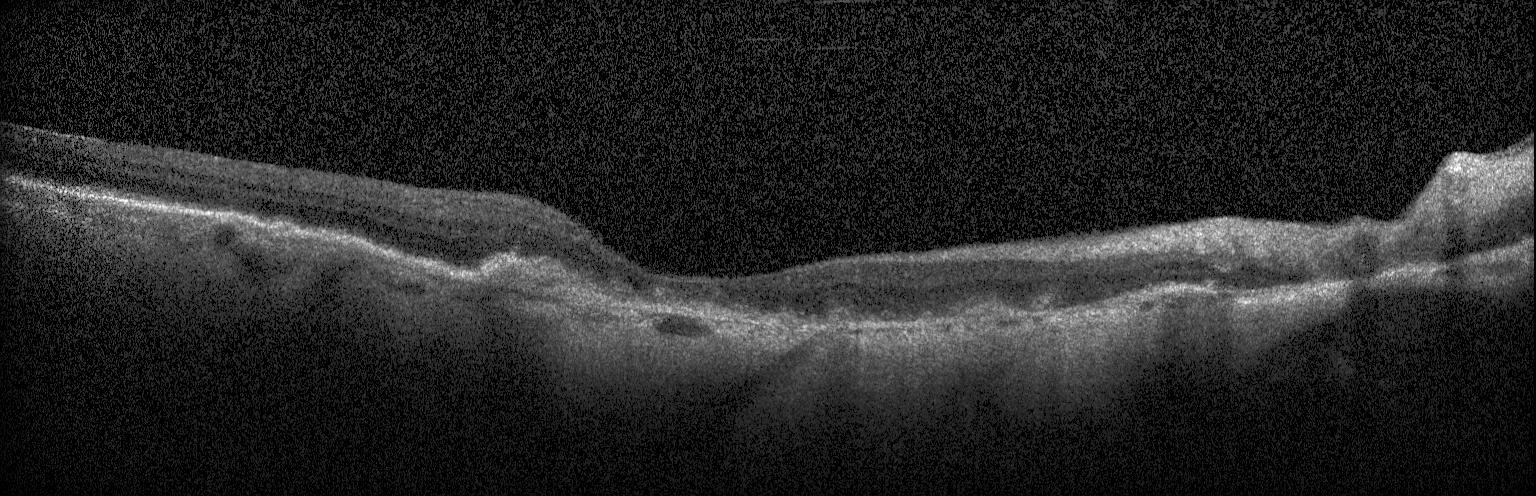
OCT B-scan. SD-OCT — The scan shows a choroidal neovascular membrane.